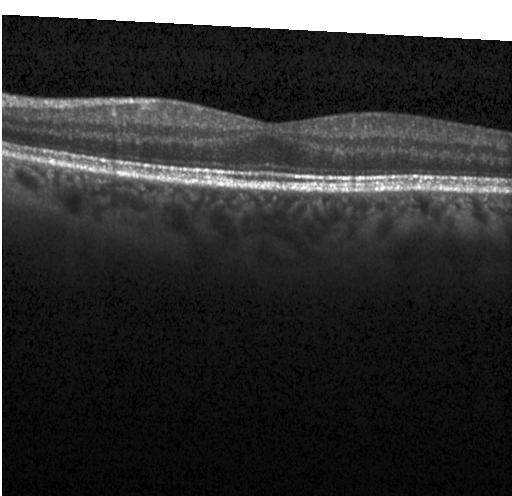

Heidelberg Spectralis OCT system; optical coherence tomography scan.
Assessment: neither CNV, DME, nor drusen.